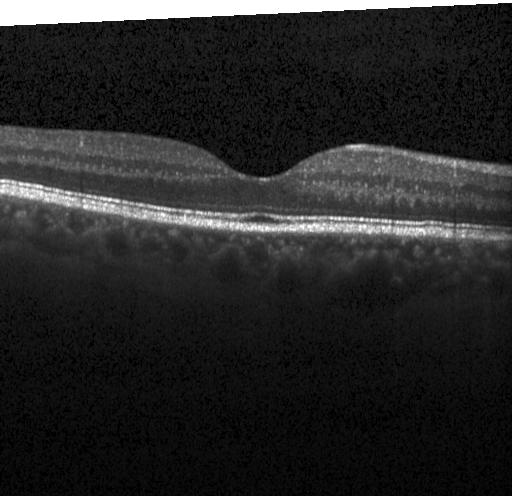

OCT B-scan
Dx: no evidence of CNV, DME, or drusen.